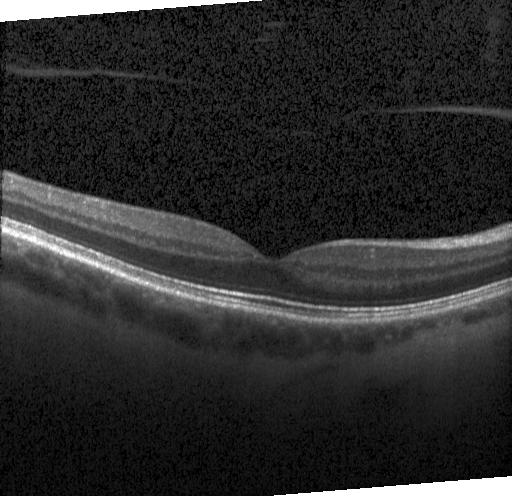

OCT B-scan showing no choroidal neovascularization, diabetic macular edema, or drusen.